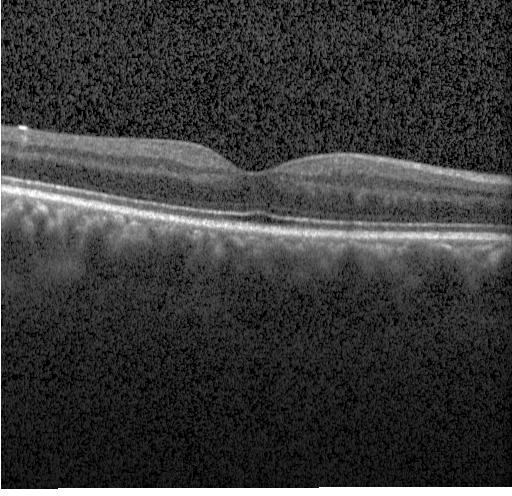
Macular OCT demonstrating no evidence of choroidal neovascularization, diabetic macular edema, or drusen.